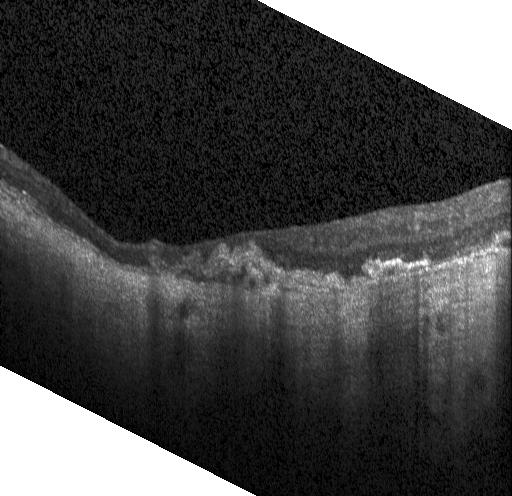

Impression: choroidal neovascularization.